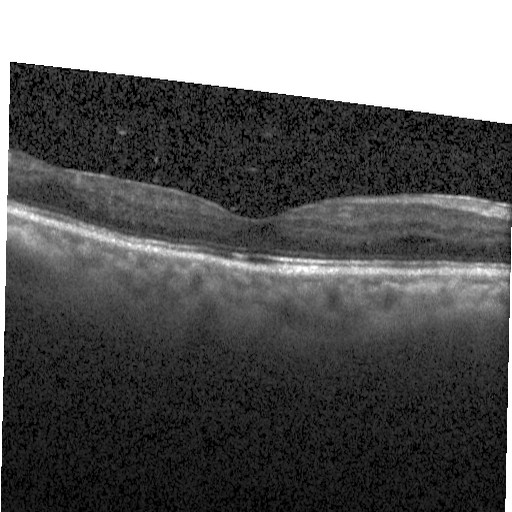 Finding: diabetic macular edema.